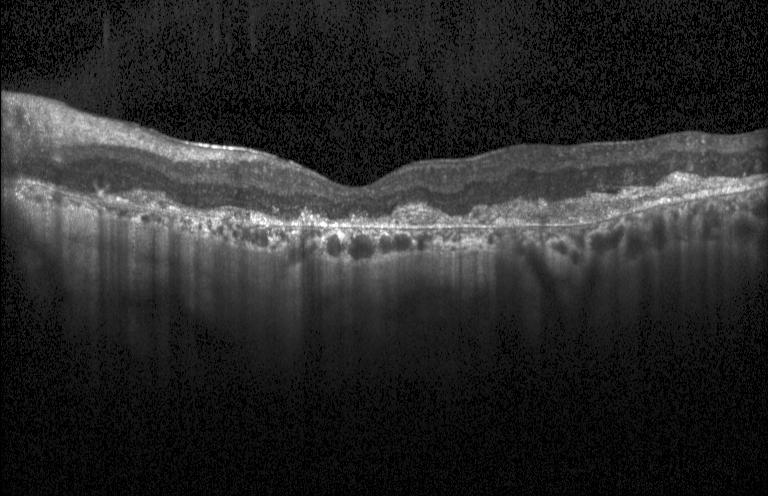

Spectral-domain OCT · Heidelberg Spectralis OCT system · centered on the fovea · OCT line scan. Diagnosis: choroidal neovascularization.